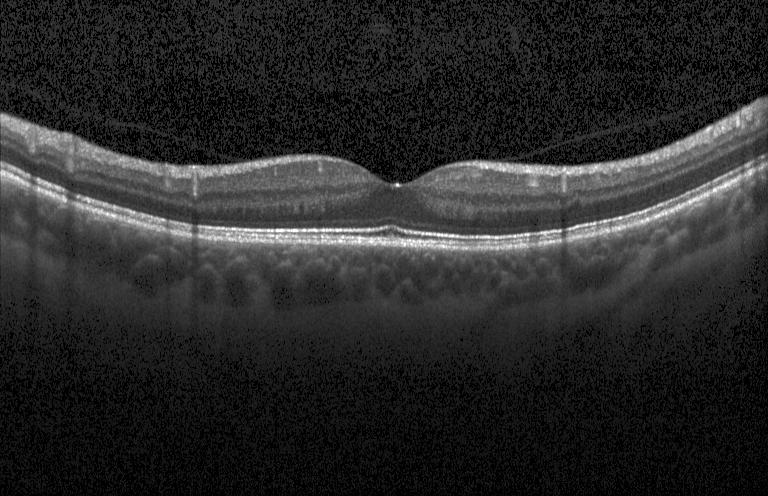

Retinal OCT cross-section. Impression: no CNV, DME, or drusen.